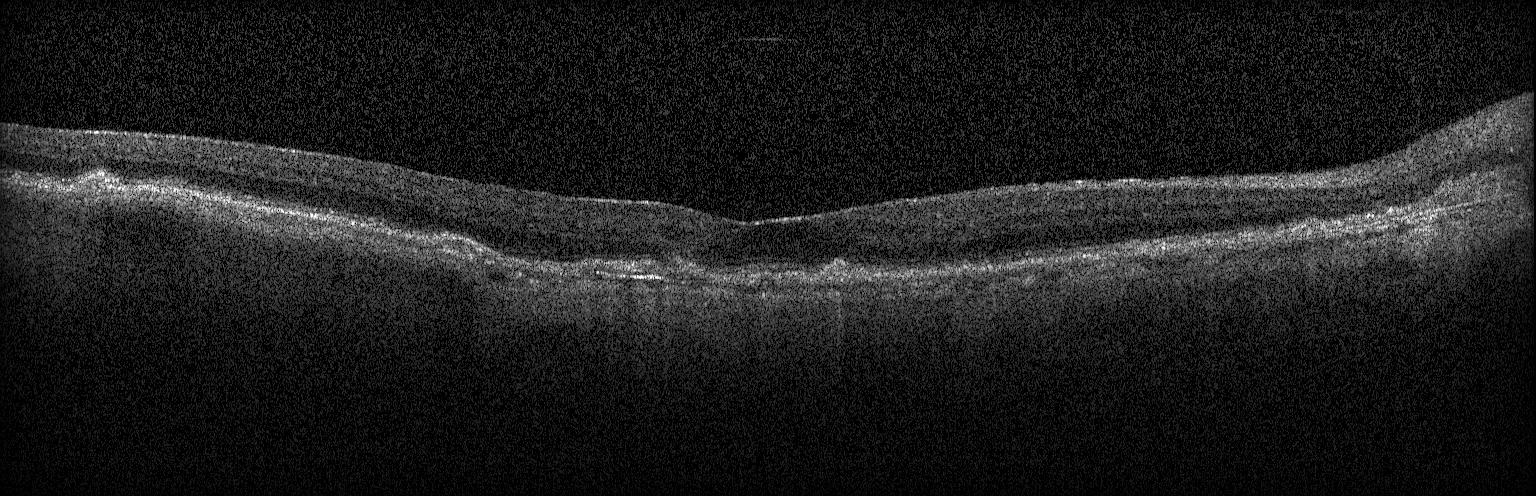

Macular OCT demonstrating a choroidal neovascular membrane.